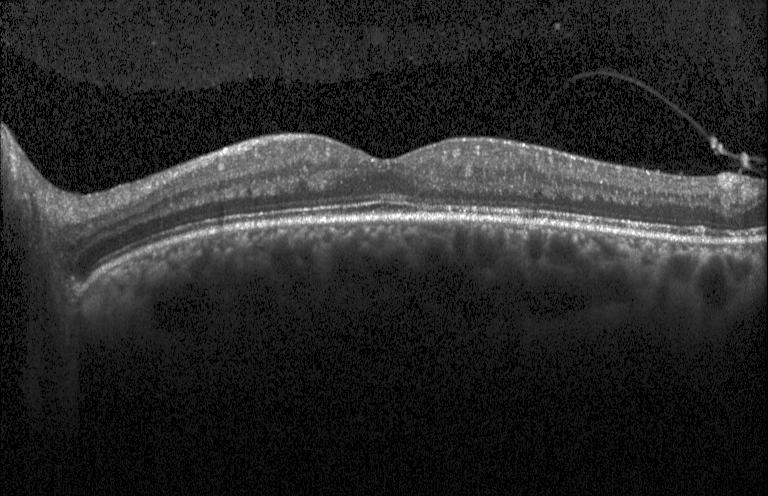 SD-OCT, retinal OCT B-scan. No CNV, no DME, and no drusen.